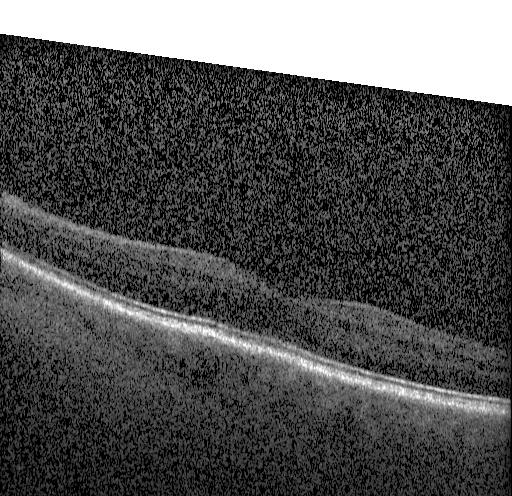 Retinal OCT cross-section. SD-OCT. Instrument: Heidelberg Spectralis. Horizontal scan through the fovea
This B-scan demonstrates neither choroidal neovascularization, diabetic macular edema, nor drusen.